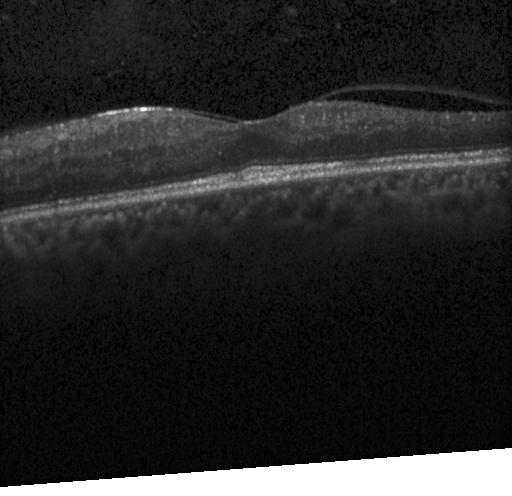

Instrument: Heidelberg Spectralis · OCT B-scan — Impression: diabetic macular edema.